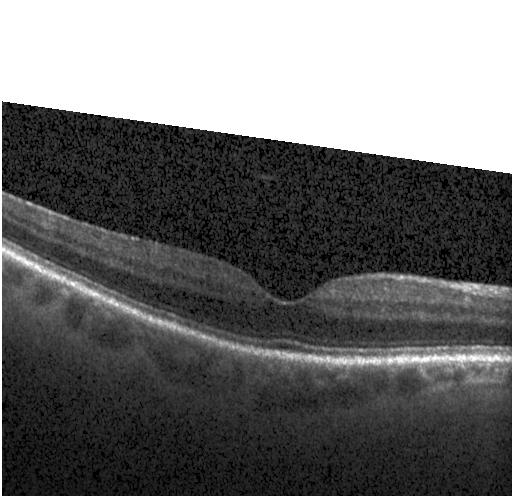

Fovea-centered; spectral-domain optical coherence tomography; retinal OCT B-scan — The scan shows neither choroidal neovascularization, diabetic macular edema, nor drusen.